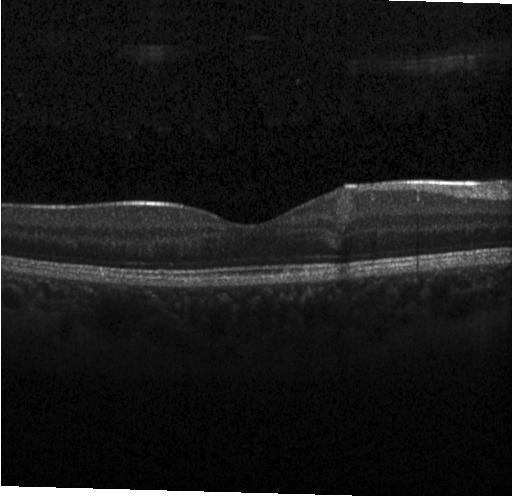 SD-OCT. Macular scan. OCT B-scan.
OCT finding: neither choroidal neovascularization, diabetic macular edema, nor drusen.